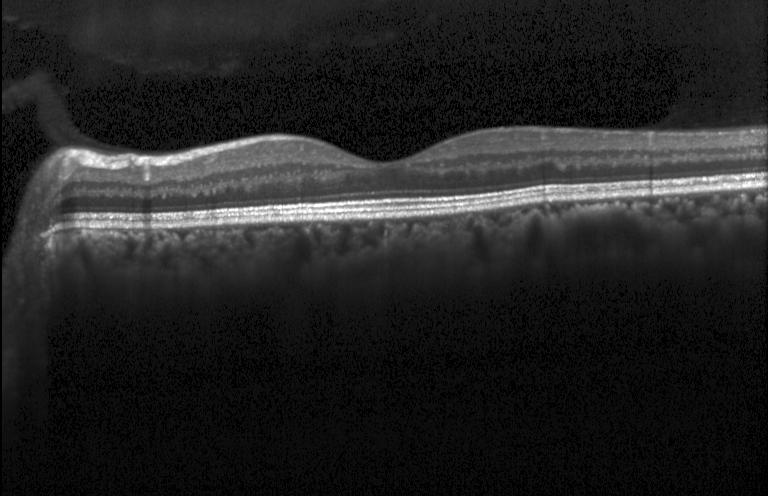 Spectral-domain optical coherence tomography. Retinal OCT cross-section — Diagnosis: neither choroidal neovascularization, diabetic macular edema, nor drusen.